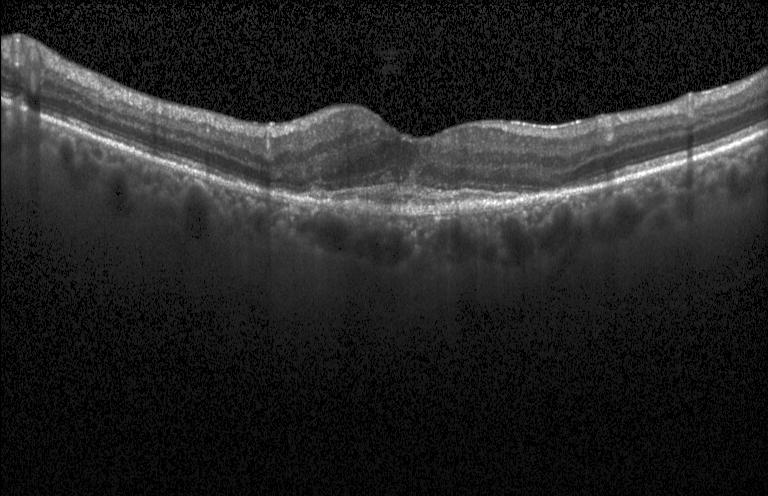 Optical coherence tomography B-scan, Heidelberg Spectralis OCT system, spectral-domain optical coherence tomography
Impression: choroidal neovascularization.